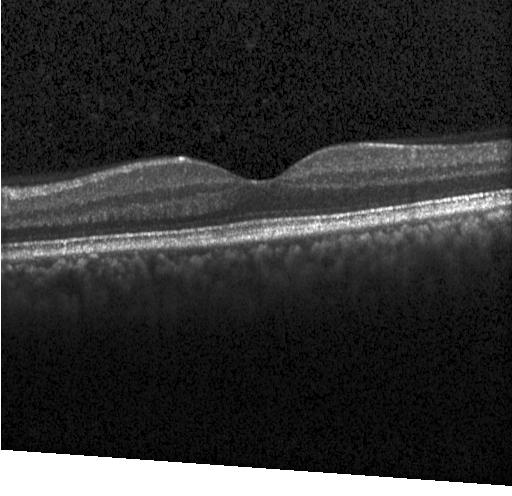

Spectral-domain optical coherence tomography. Retinal OCT B-scan. Instrument: Heidelberg Spectralis — Neither choroidal neovascularization, diabetic macular edema, nor drusen.